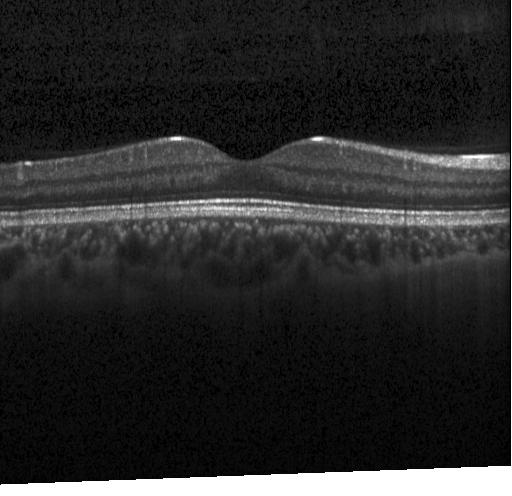

Retinal OCT cross-section · centered on the fovea · SD-OCT — This B-scan demonstrates neither choroidal neovascularization, diabetic macular edema, nor drusen.